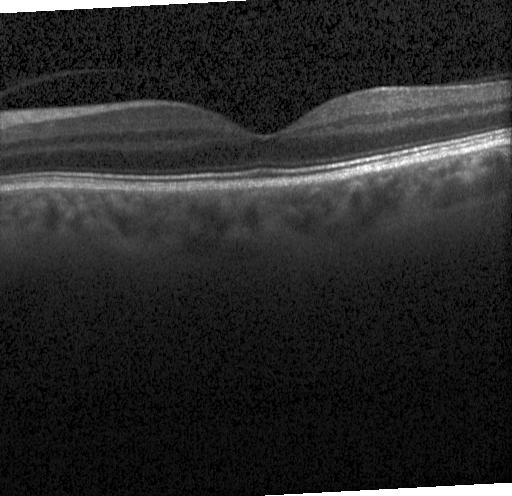
OCT B-scan showing no evidence of CNV, DME, or drusen.